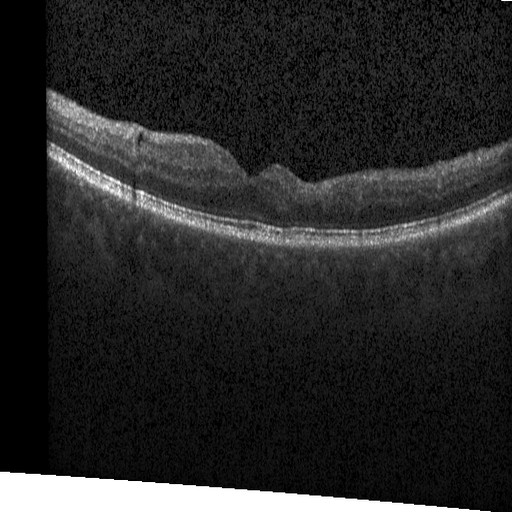 Dx: DME.